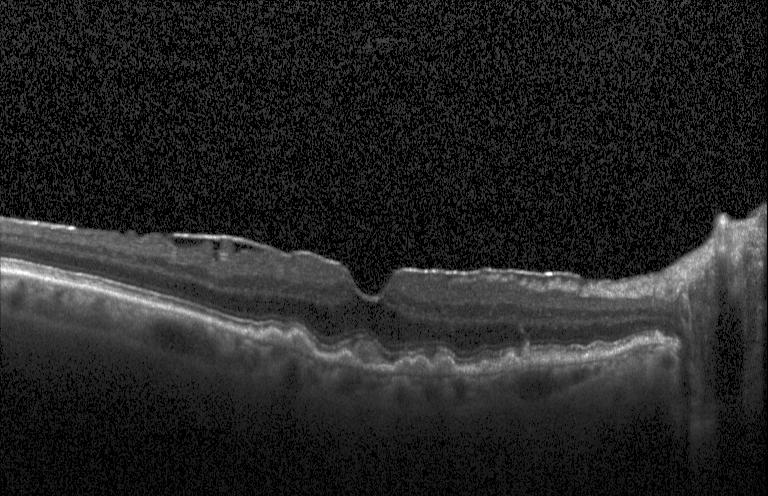 Macular scan; optical coherence tomography scan; acquired on a Heidelberg Spectralis; spectral-domain optical coherence tomography. Impression: sub-RPE drusenoid deposits.